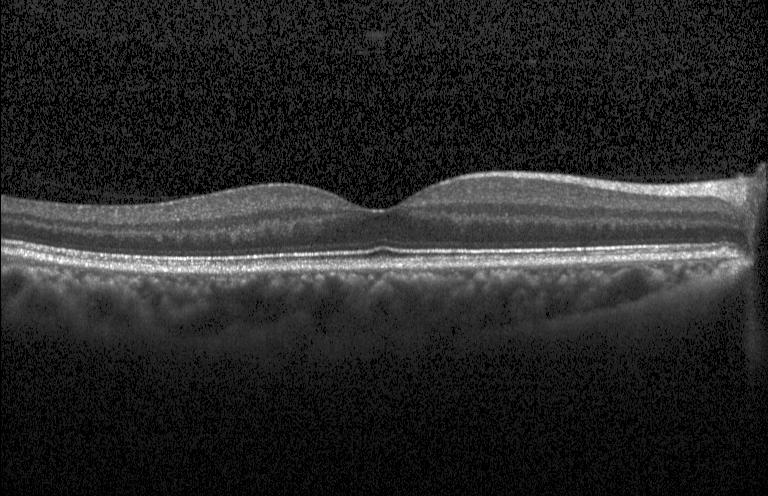 OCT finding: no evidence of choroidal neovascularization, diabetic macular edema, or drusen.